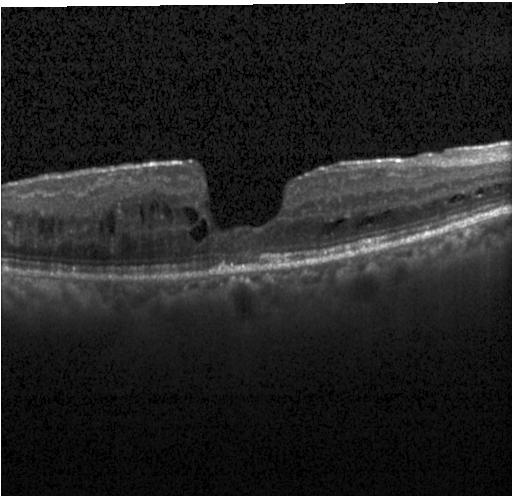

OCT B-scan
Impression: diabetic macular edema (DME).